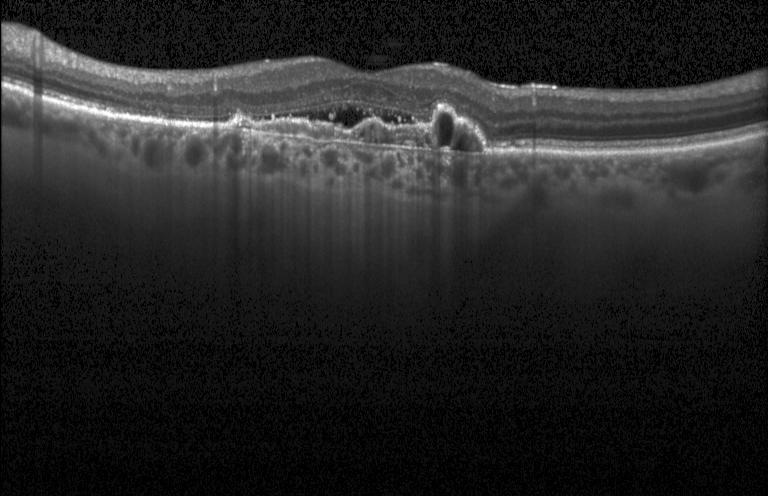
OCT line scan; macular scan; instrument: Heidelberg Spectralis — OCT finding: choroidal neovascularization.